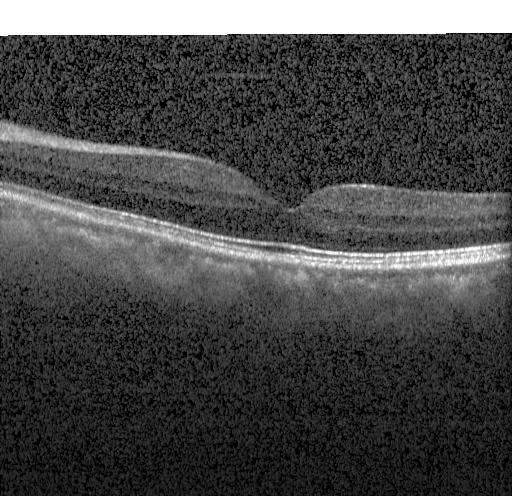

Retinal OCT cross-section. Instrument: Heidelberg Spectralis. Spectral-domain optical coherence tomography. Horizontal scan through the fovea
Dx: no choroidal neovascularization, diabetic macular edema, or drusen.